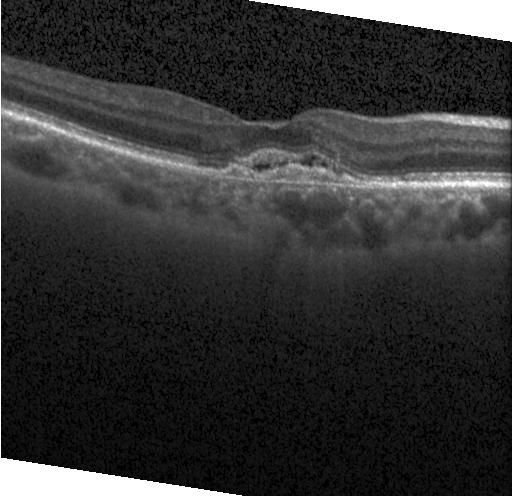

Finding: a choroidal neovascular membrane.